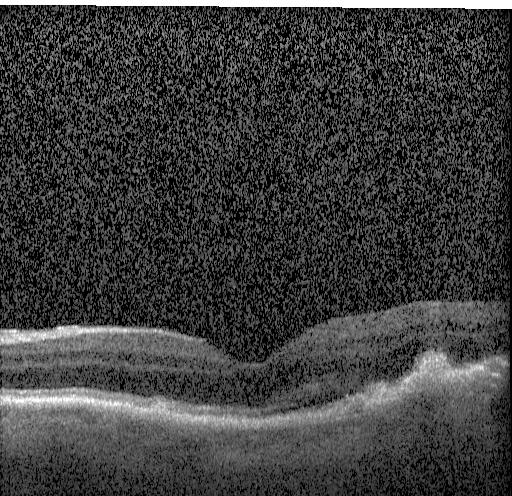
Heidelberg Spectralis OCT system; horizontal scan through the fovea; SD-OCT; optical coherence tomography B-scan — Finding: choroidal neovascularization (CNV).